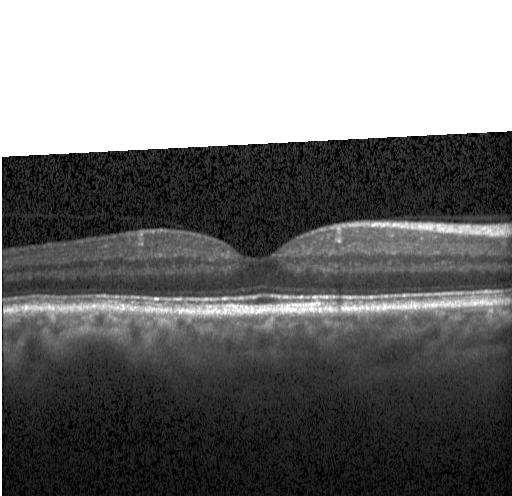

Finding: no choroidal neovascularization, diabetic macular edema, or drusen.